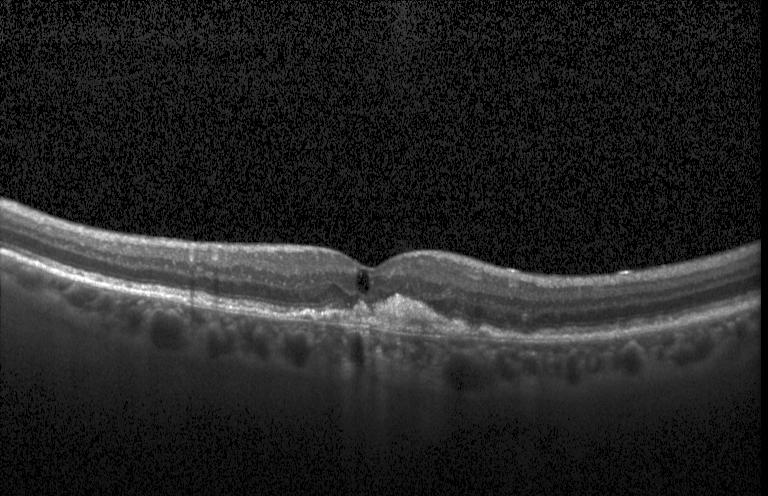
Retinal OCT cross-section · SD-OCT. Dx: CNV.